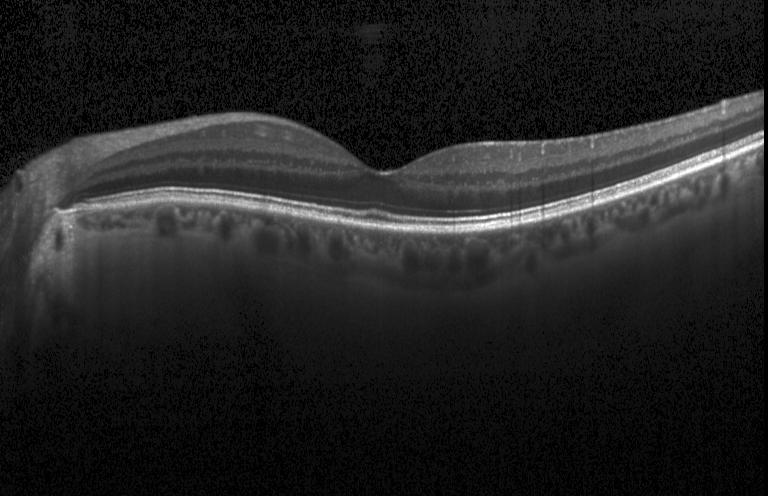 Instrument: Heidelberg Spectralis · OCT line scan · spectral-domain optical coherence tomography · through the macula. Finding: neither choroidal neovascularization, diabetic macular edema, nor drusen.